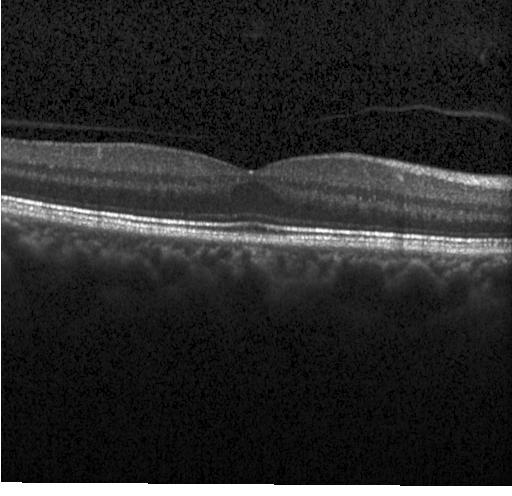
Macular OCT demonstrating no choroidal neovascularization, no diabetic macular edema, and no drusen.